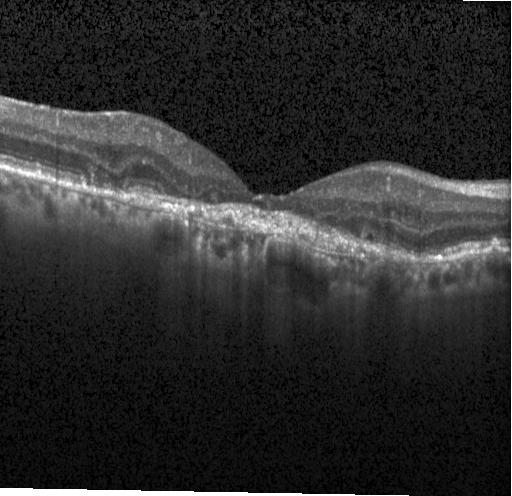 Retinal OCT cross-section — The scan shows a choroidal neovascular membrane.